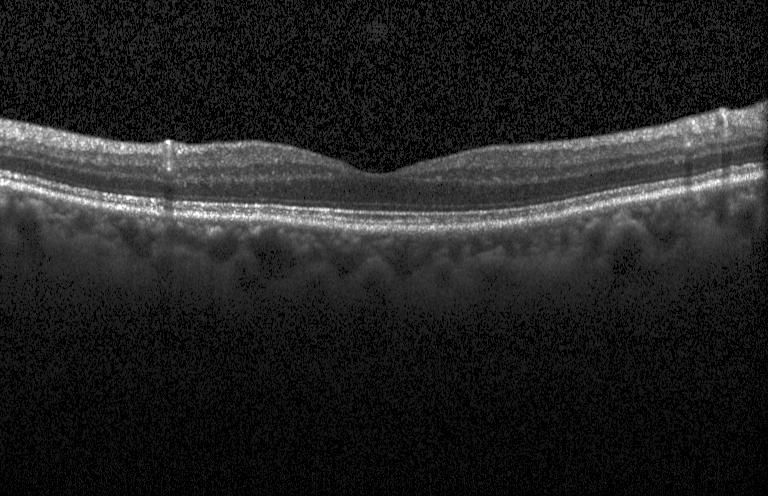 Impression: no CNV, no DME, and no drusen.